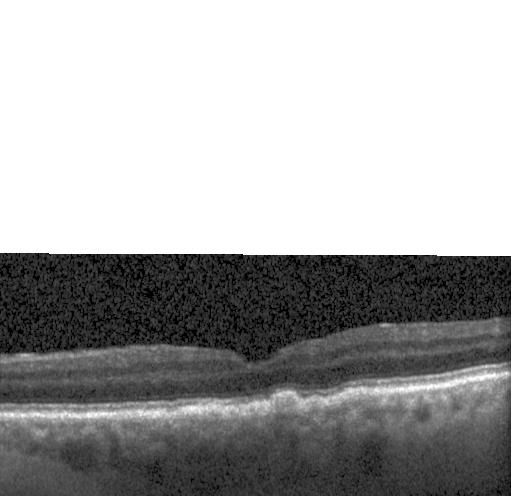

Spectral-domain optical coherence tomography · retinal OCT B-scan
Impression: sub-RPE drusenoid deposits.